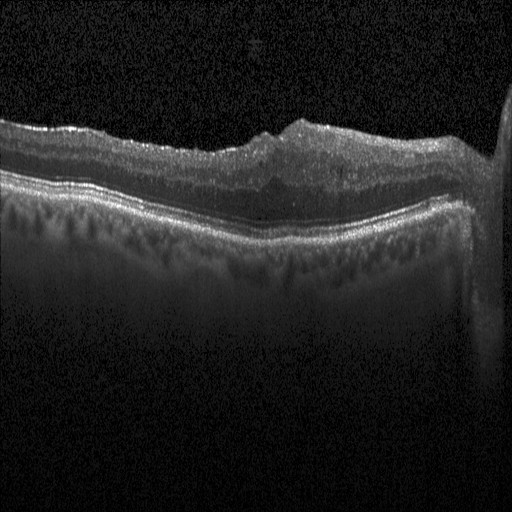

Impression: diabetic macular edema (DME).